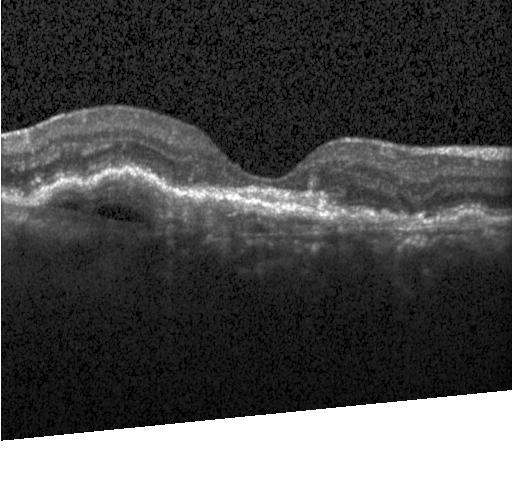
OCT line scan
Impression: choroidal neovascularization (CNV).